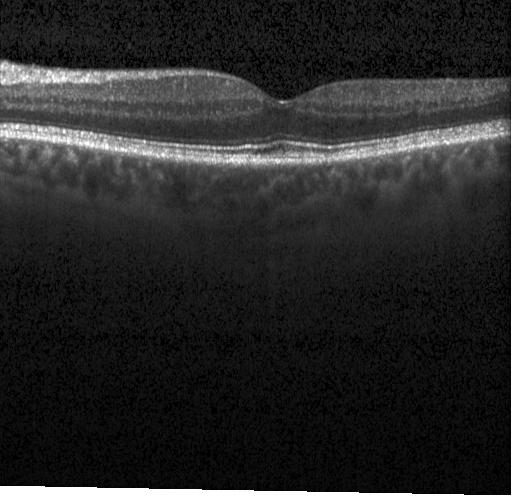

Retinal OCT cross-section showing neither choroidal neovascularization, diabetic macular edema, nor drusen.